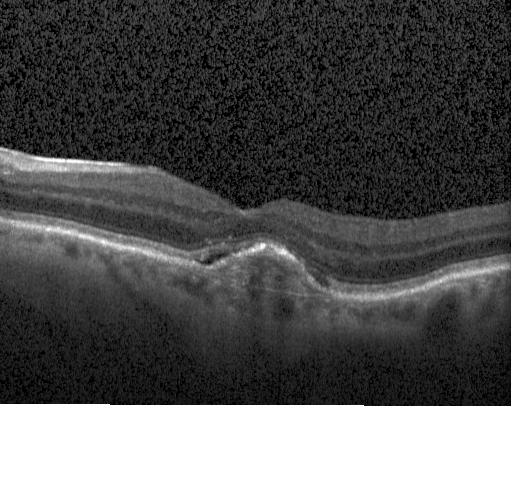 Optical coherence tomography B-scan · spectral-domain optical coherence tomography. Finding: choroidal neovascularization (CNV).